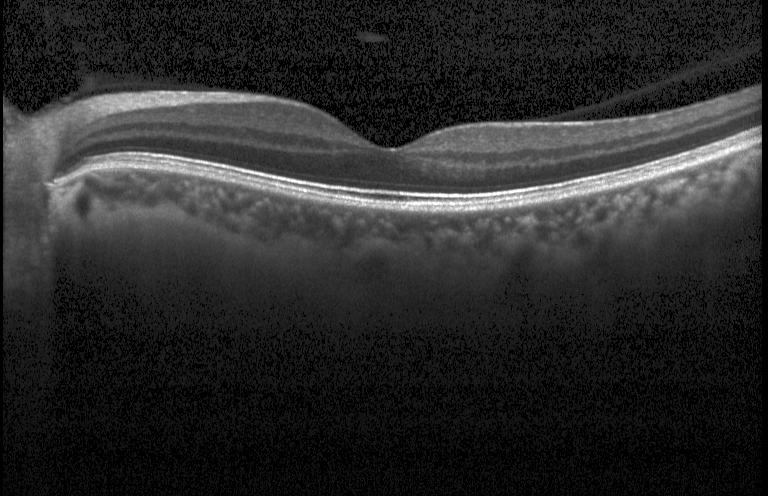

Diagnosis: no evidence of choroidal neovascularization, diabetic macular edema, or drusen.